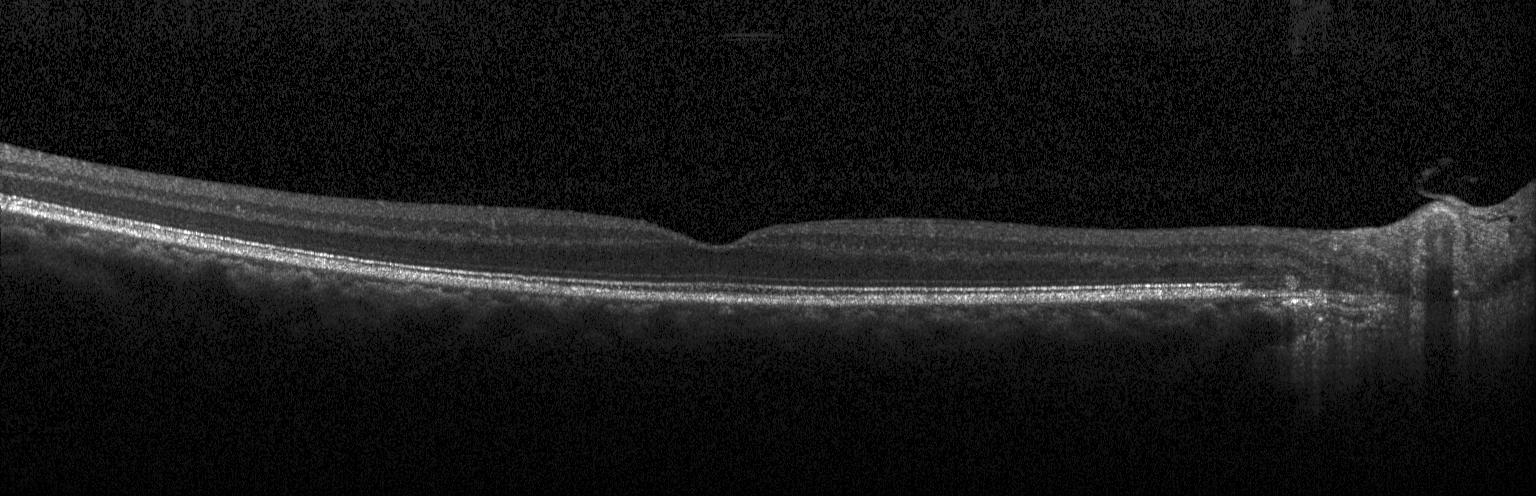
Retinal OCT cross-section showing no choroidal neovascularization, diabetic macular edema, or drusen.